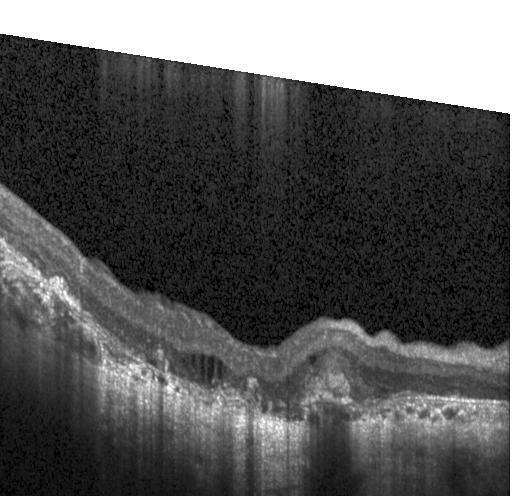
OCT B-scan. Finding: CNV.